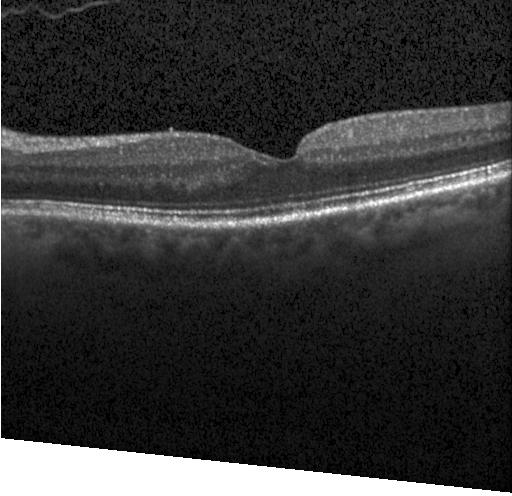 No CNV, DME, or drusen.